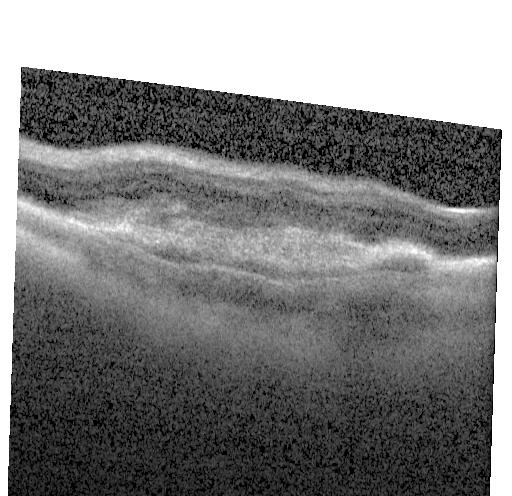 SD-OCT. OCT line scan. Acquired on a Heidelberg Spectralis. Horizontal scan through the fovea — Impression: choroidal neovascularization.